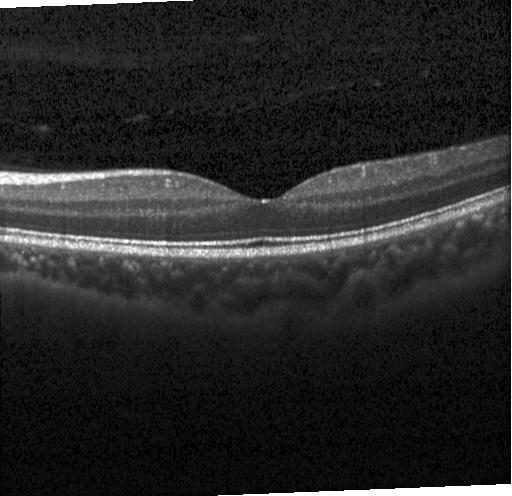
SD-OCT. OCT B-scan
Finding: neither CNV, DME, nor drusen.